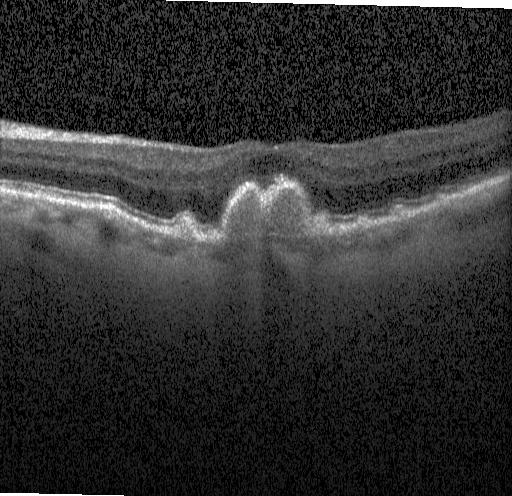
Retinal OCT cross-section
The scan shows drusen.